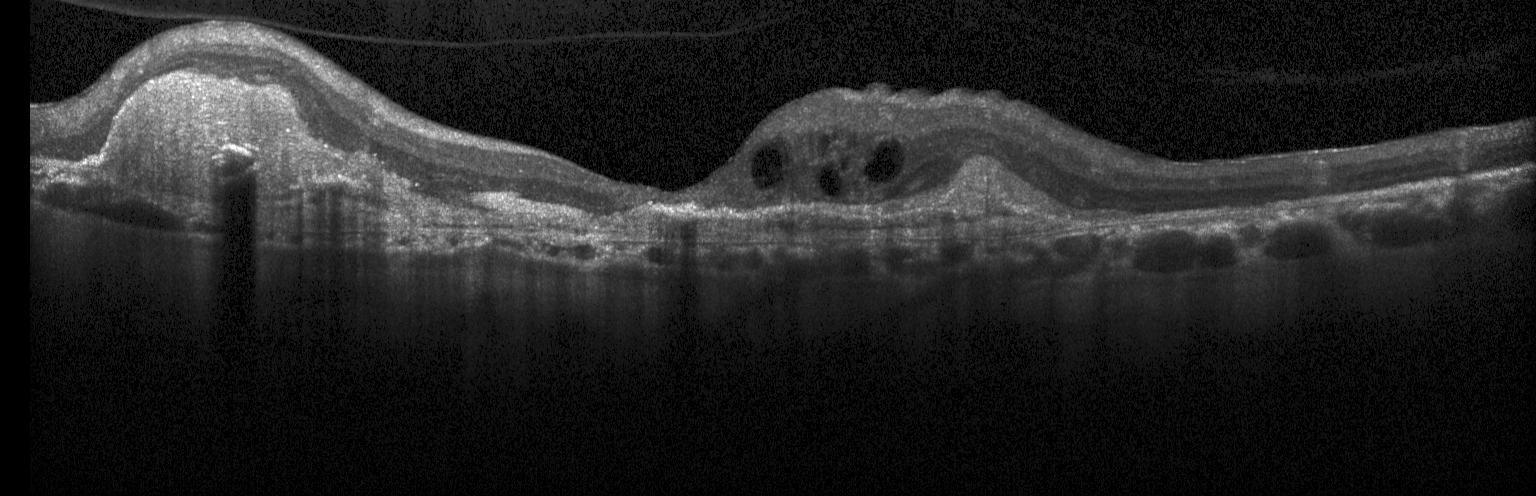 OCT line scan
This B-scan demonstrates a choroidal neovascular membrane.